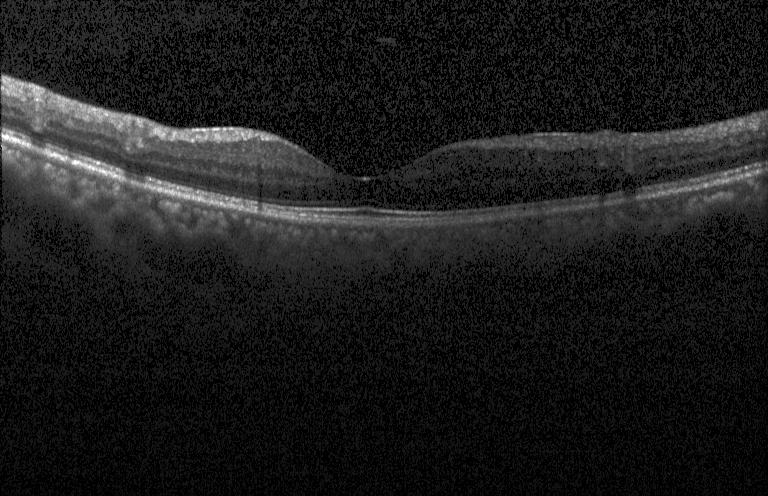

Impression: neither choroidal neovascularization, diabetic macular edema, nor drusen.